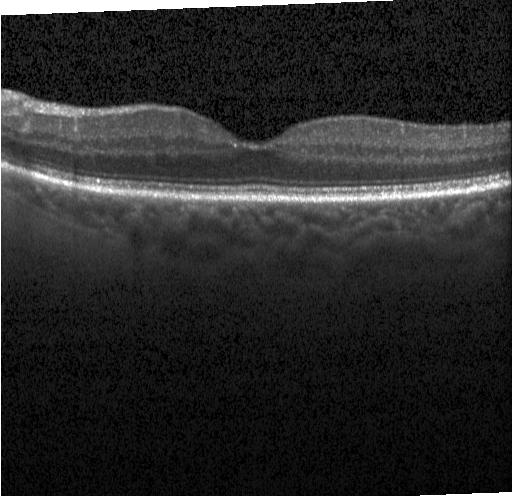

Diagnosis: no CNV, no DME, and no drusen.